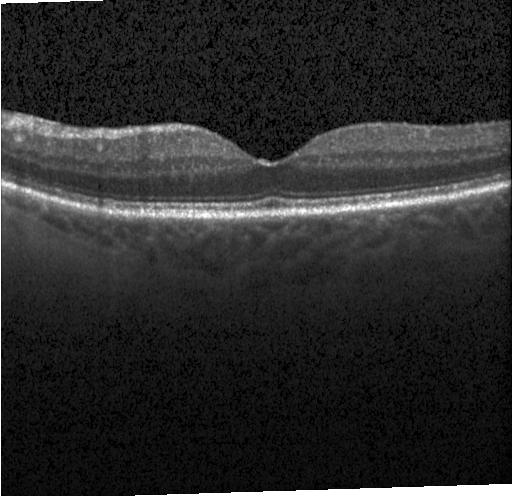 Retinal OCT cross-section showing no evidence of choroidal neovascularization, diabetic macular edema, or drusen.